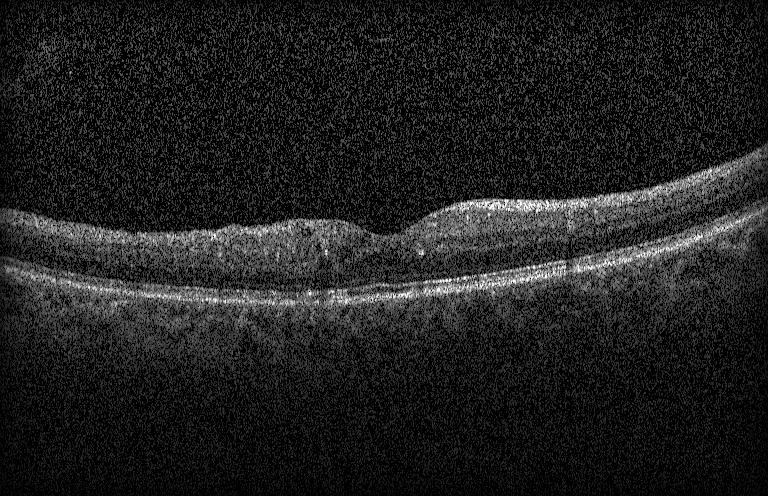 Assessment: no choroidal neovascularization, no diabetic macular edema, and no drusen.